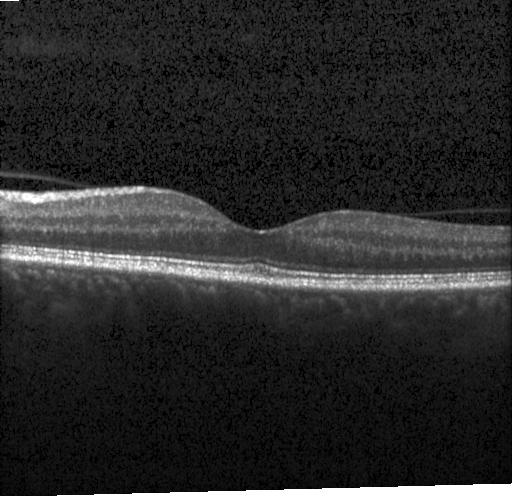 This B-scan demonstrates no choroidal neovascularization, no diabetic macular edema, and no drusen.